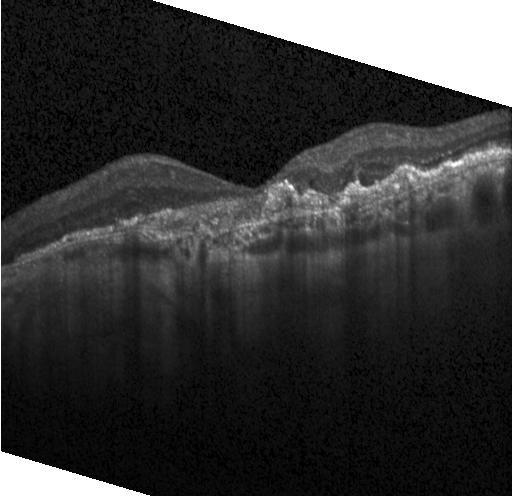 OCT scan showing choroidal neovascularization.